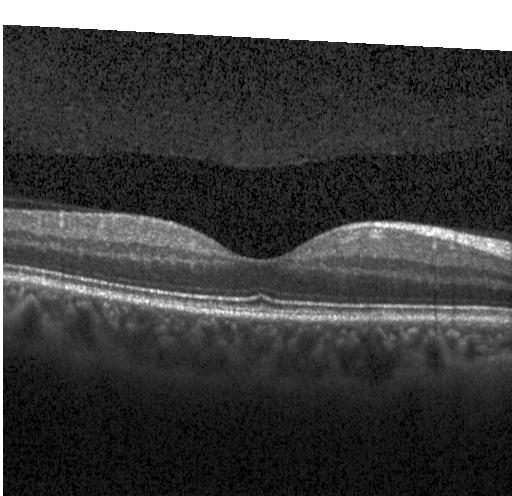

Optical coherence tomography B-scan; SD-OCT
Impression: no choroidal neovascularization, no diabetic macular edema, and no drusen.